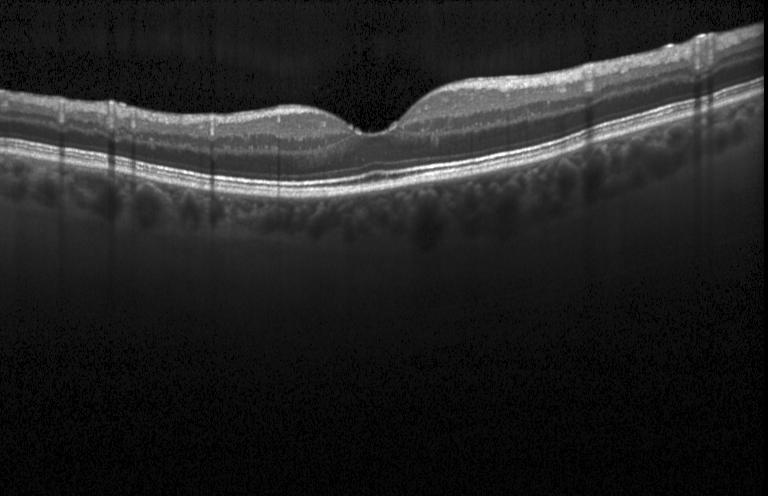

Dx: no evidence of CNV, DME, or drusen.